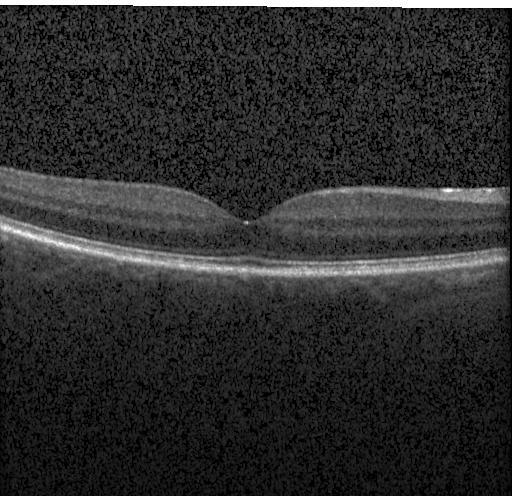

Macular OCT demonstrating no CNV, no DME, and no drusen.